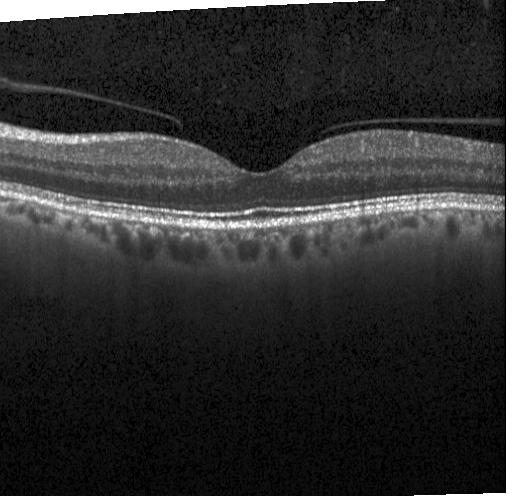

Fovea-centered · spectral-domain optical coherence tomography · optical coherence tomography B-scan · acquired on a Heidelberg Spectralis
Assessment: neither choroidal neovascularization, diabetic macular edema, nor drusen.